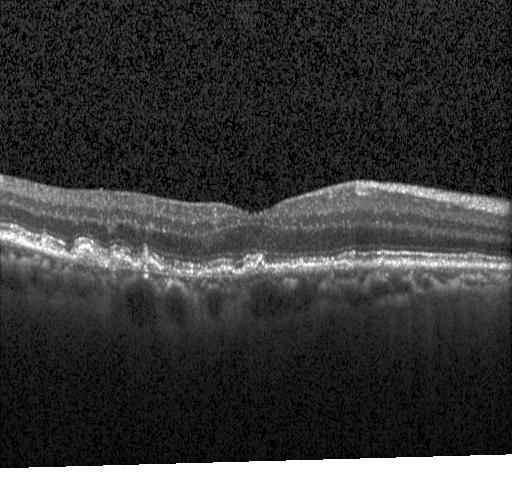 Macular OCT demonstrating multiple drusen.